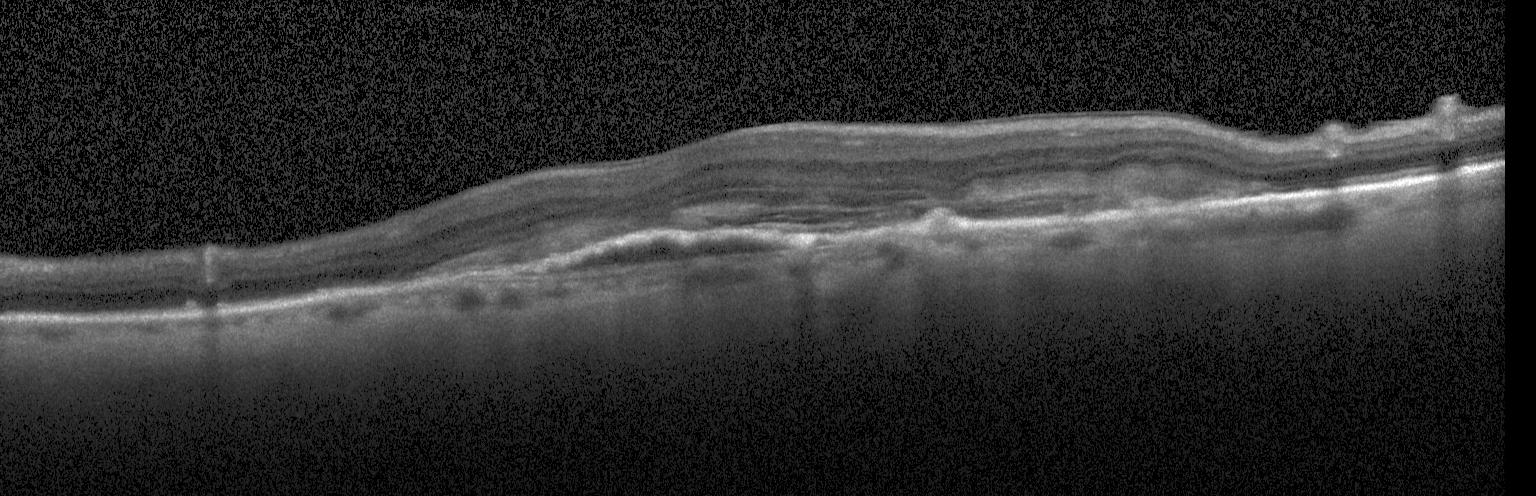 Acquired on a Heidelberg Spectralis · OCT line scan · fovea-centered · spectral-domain OCT.
Diagnosis: choroidal neovascularization (CNV).